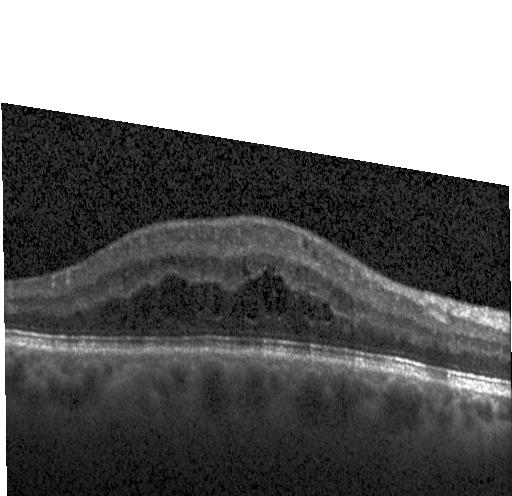
Finding: diabetic macular edema (DME).